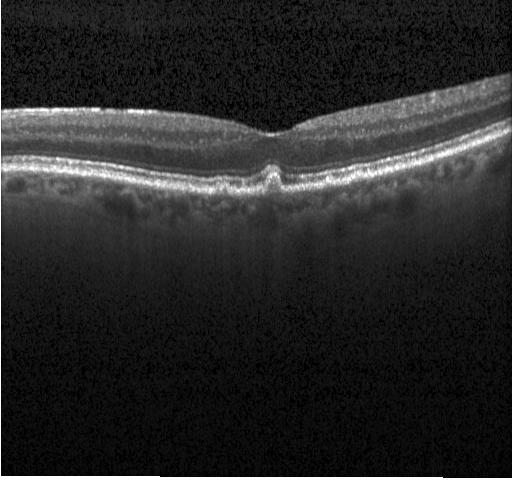
Macular OCT demonstrating drusen.